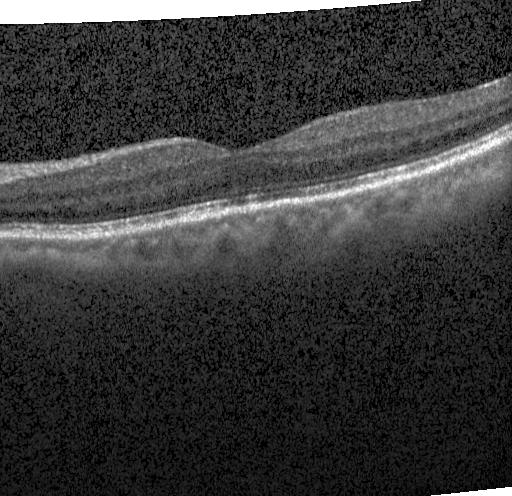
Macular OCT: no choroidal neovascularization, no diabetic macular edema, and no drusen.